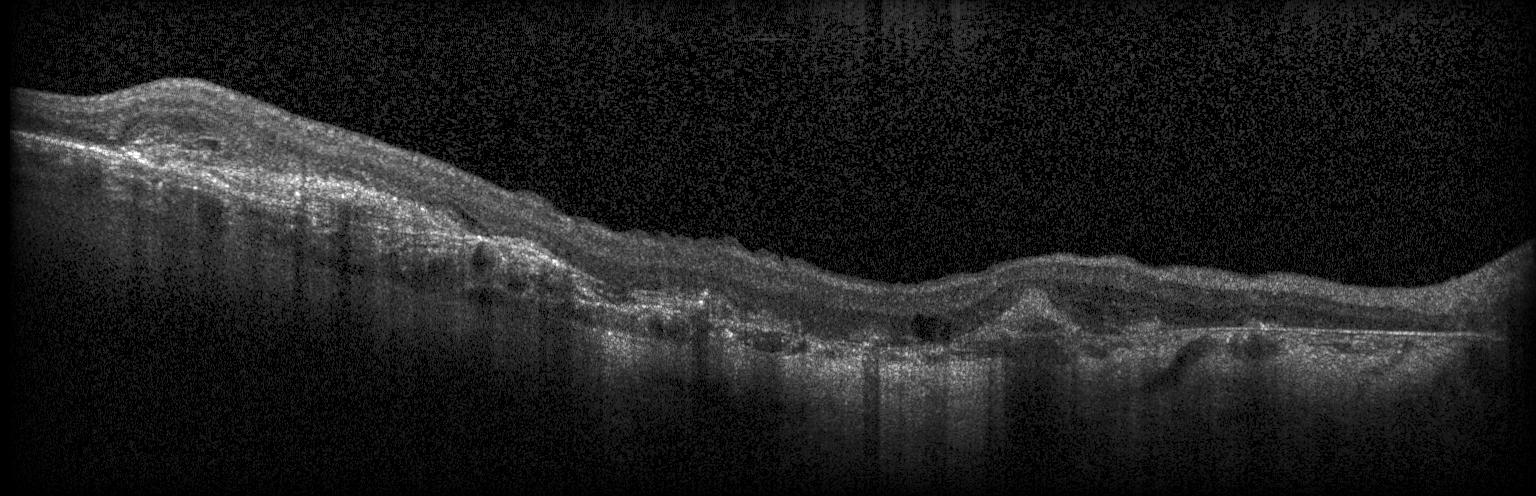
Optical coherence tomography scan. Instrument: Heidelberg Spectralis. Through the macula. Spectral-domain optical coherence tomography — Macular OCT: choroidal neovascularization.